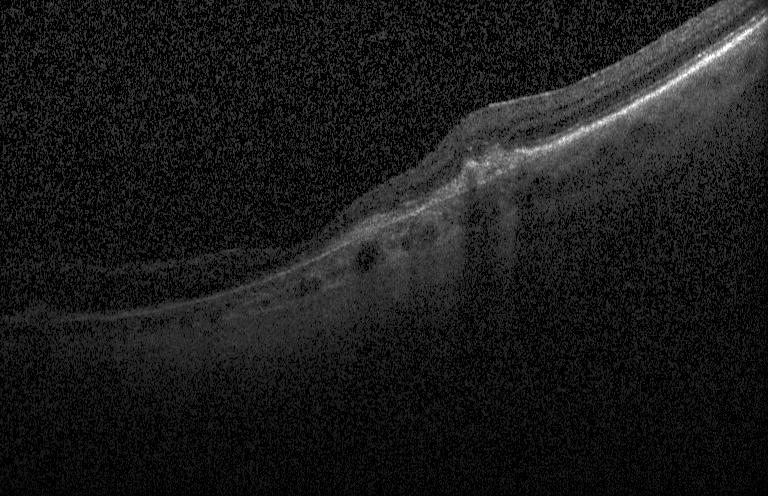 Optical coherence tomography scan.
Finding: a choroidal neovascular membrane.